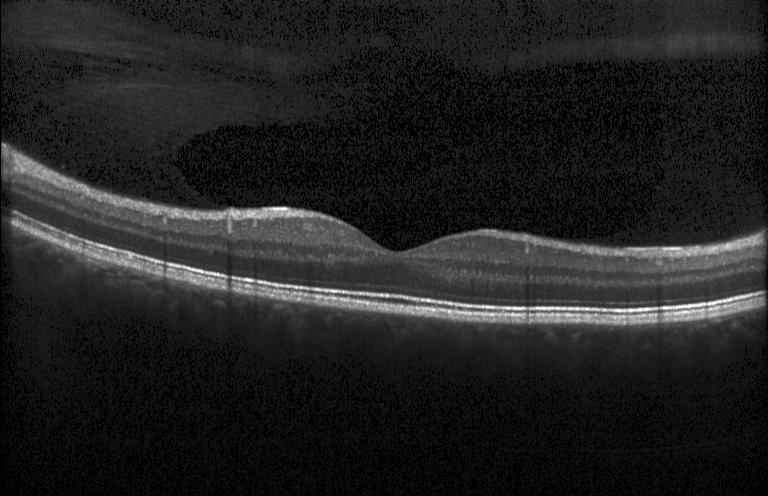 Spectral-domain OCT B-scan: no evidence of CNV, DME, or drusen.